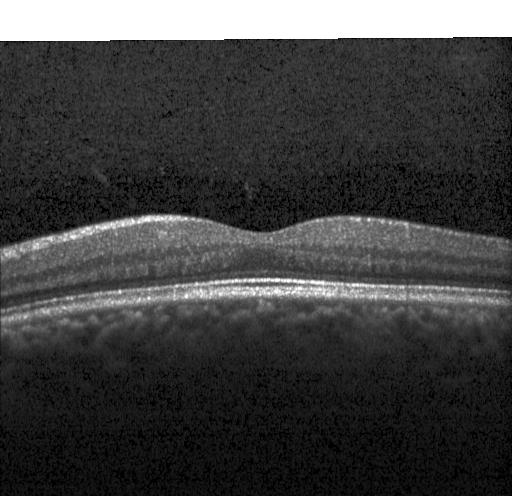 Spectral-domain OCT B-scan: no evidence of CNV, DME, or drusen.